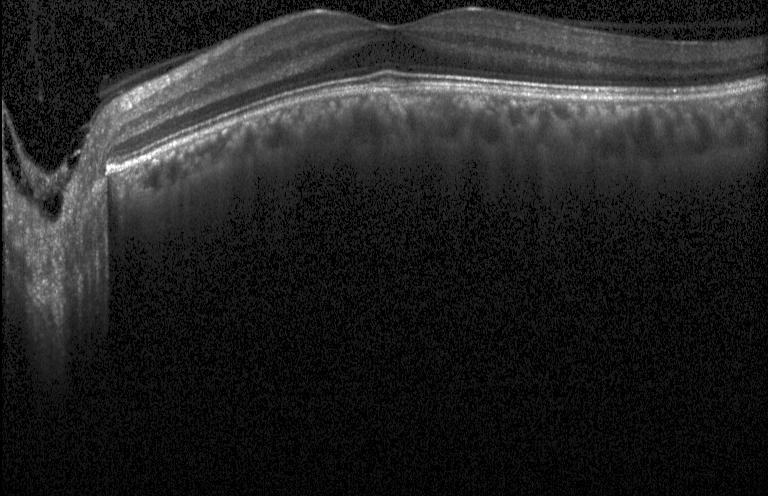
Centered on the fovea · acquired on a Heidelberg Spectralis · optical coherence tomography B-scan · spectral-domain optical coherence tomography.
Impression: no evidence of choroidal neovascularization, diabetic macular edema, or drusen.